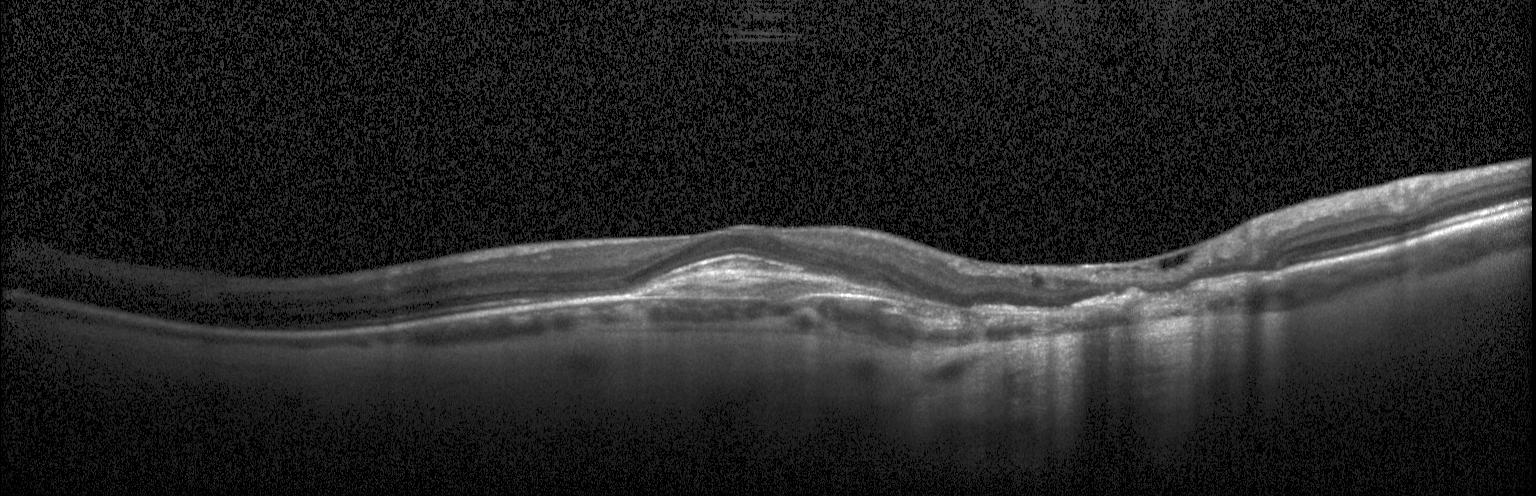
CNV.